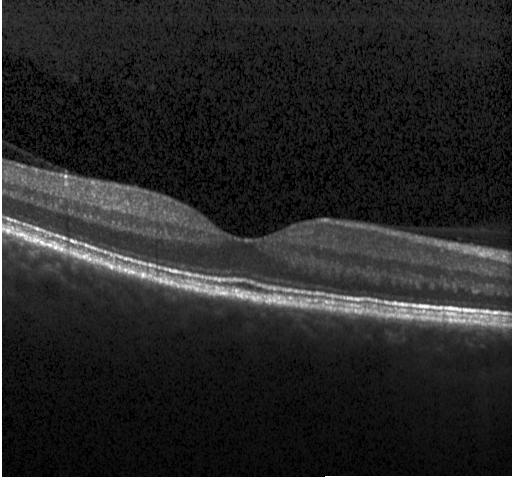

Instrument: Heidelberg Spectralis · optical coherence tomography B-scan · SD-OCT — Finding: no evidence of choroidal neovascularization, diabetic macular edema, or drusen.